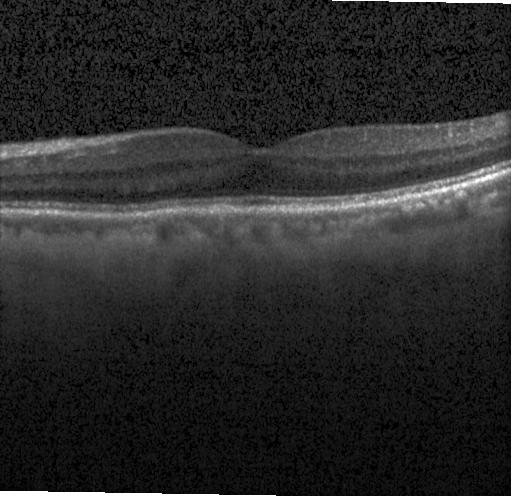

Dx: neither choroidal neovascularization, diabetic macular edema, nor drusen.